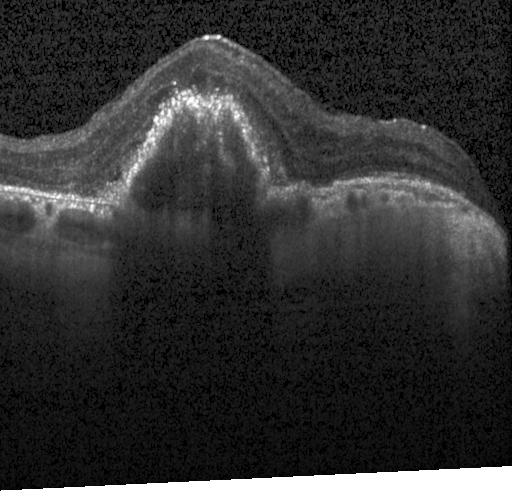 Centered on the fovea. Acquired on a Heidelberg Spectralis. OCT line scan — This B-scan demonstrates a choroidal neovascular membrane.